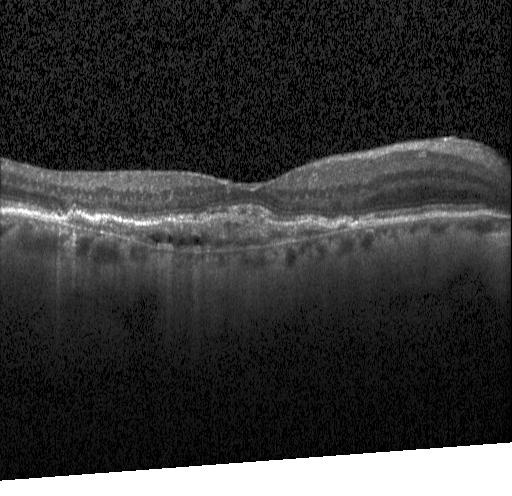 Assessment: CNV.